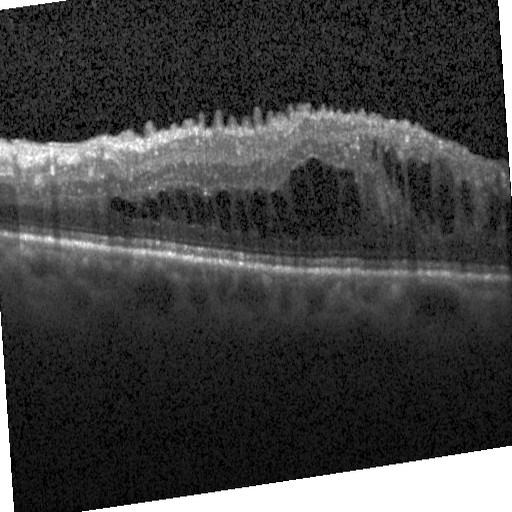

Retinal OCT cross-section · through the macula.
Impression: diabetic macular edema.